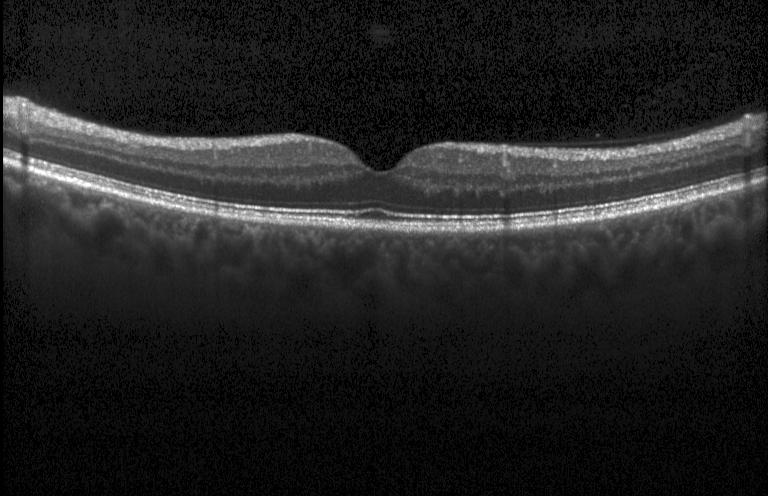
Impression: no evidence of CNV, DME, or drusen.